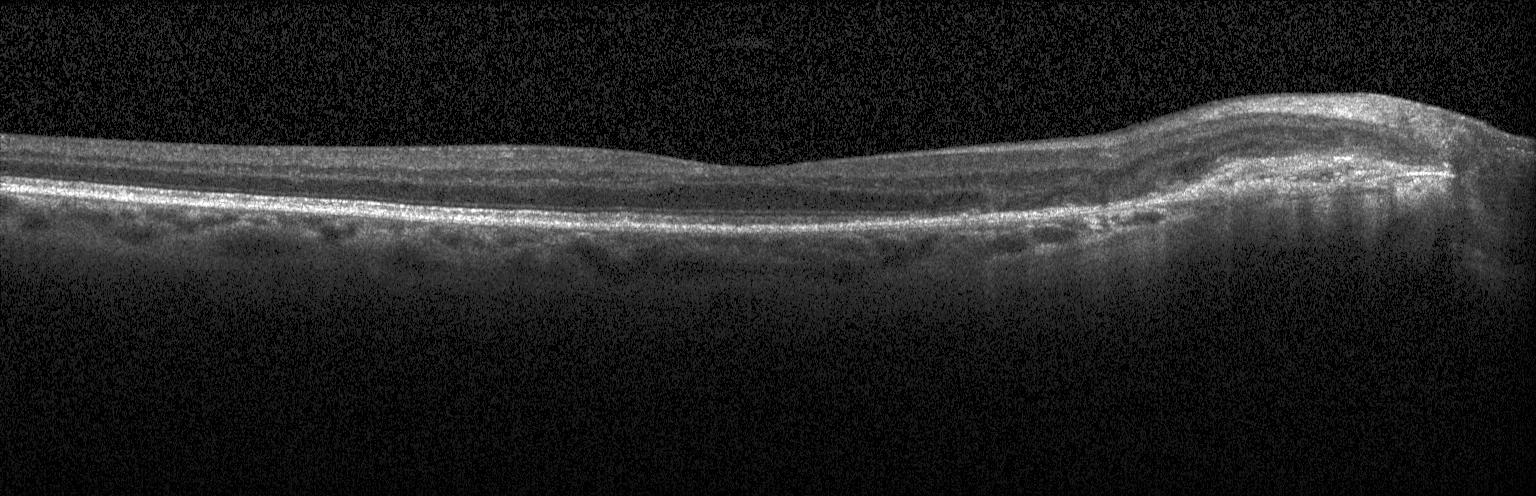 Optical coherence tomography B-scan
Choroidal neovascularization (CNV).